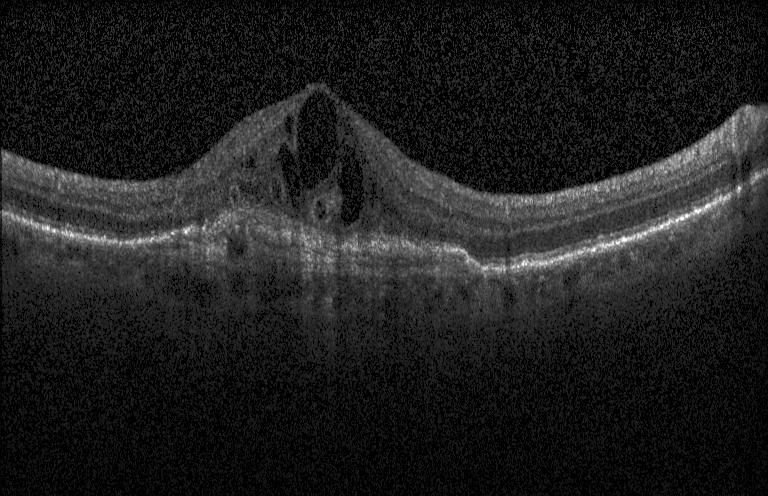
Macular OCT demonstrating choroidal neovascularization.